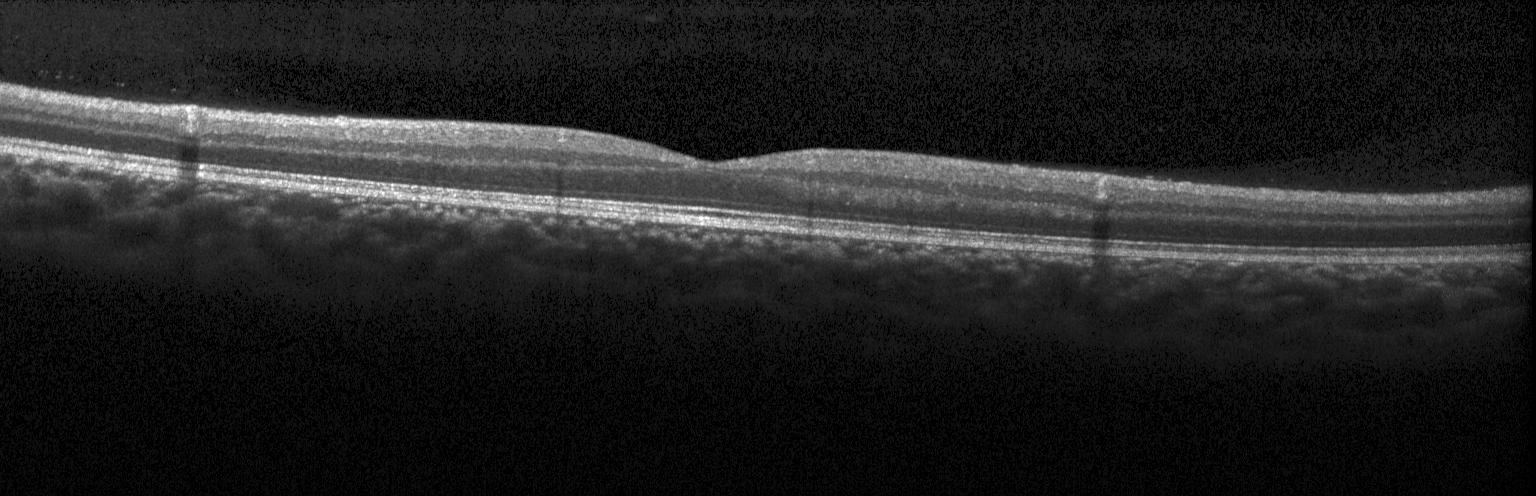 Finding: no choroidal neovascularization, diabetic macular edema, or drusen.